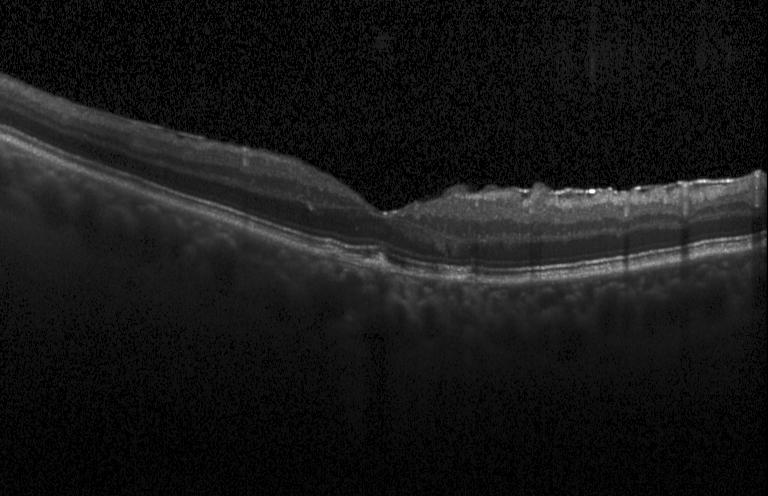

Optical coherence tomography B-scan
OCT finding: sub-RPE drusenoid deposits.